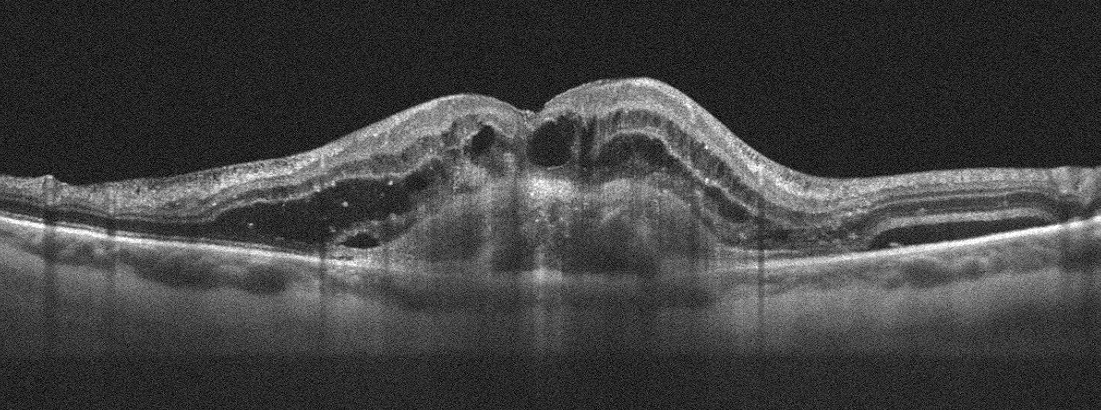 Diagnosis: AMD.